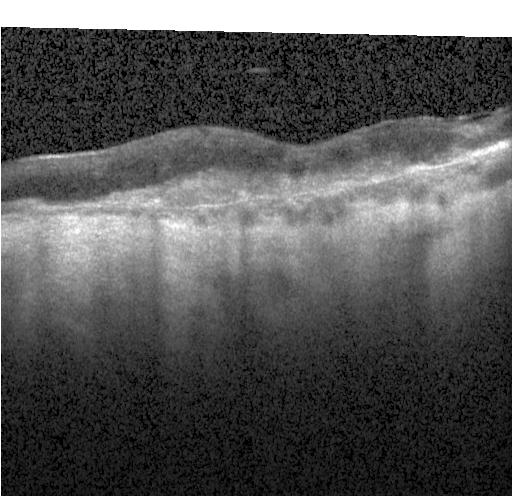

Optical coherence tomography B-scan; acquired on a Heidelberg Spectralis; fovea-centered — Assessment: a choroidal neovascular membrane.